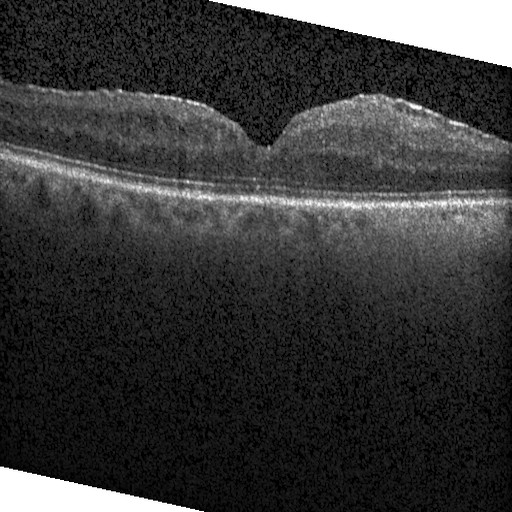

OCT B-scan. Acquired on a Heidelberg Spectralis — Assessment: diabetic macular edema (DME).